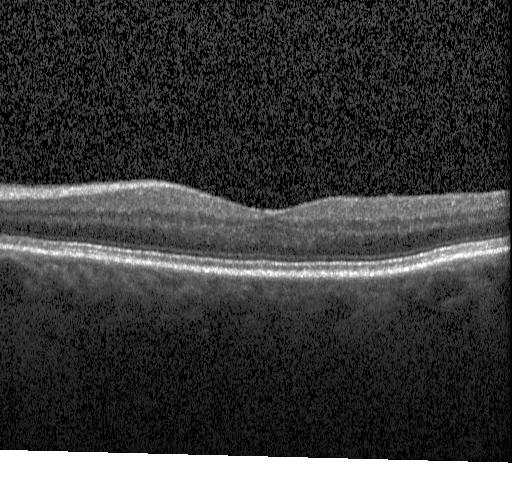

Horizontal scan through the fovea; acquired on a Heidelberg Spectralis; OCT line scan. OCT finding: no evidence of choroidal neovascularization, diabetic macular edema, or drusen.